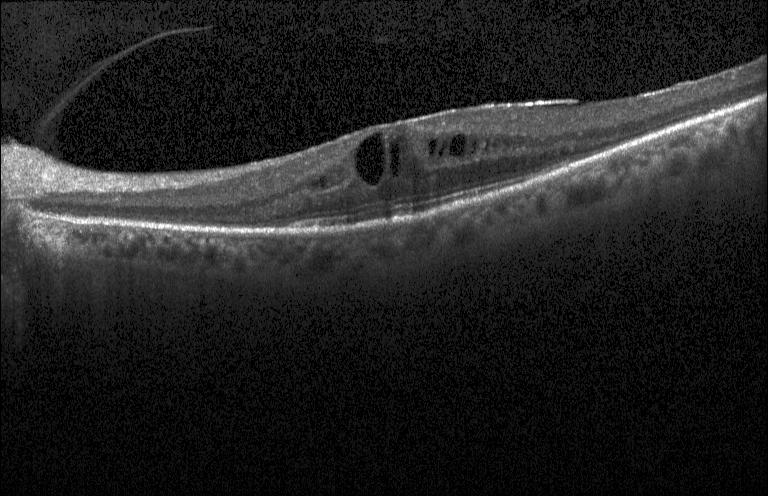

Heidelberg Spectralis OCT system, optical coherence tomography scan. Impression: diabetic macular edema.